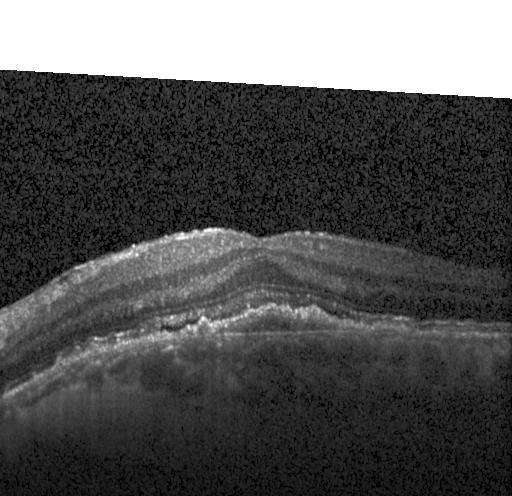 Macular OCT: a choroidal neovascular membrane.